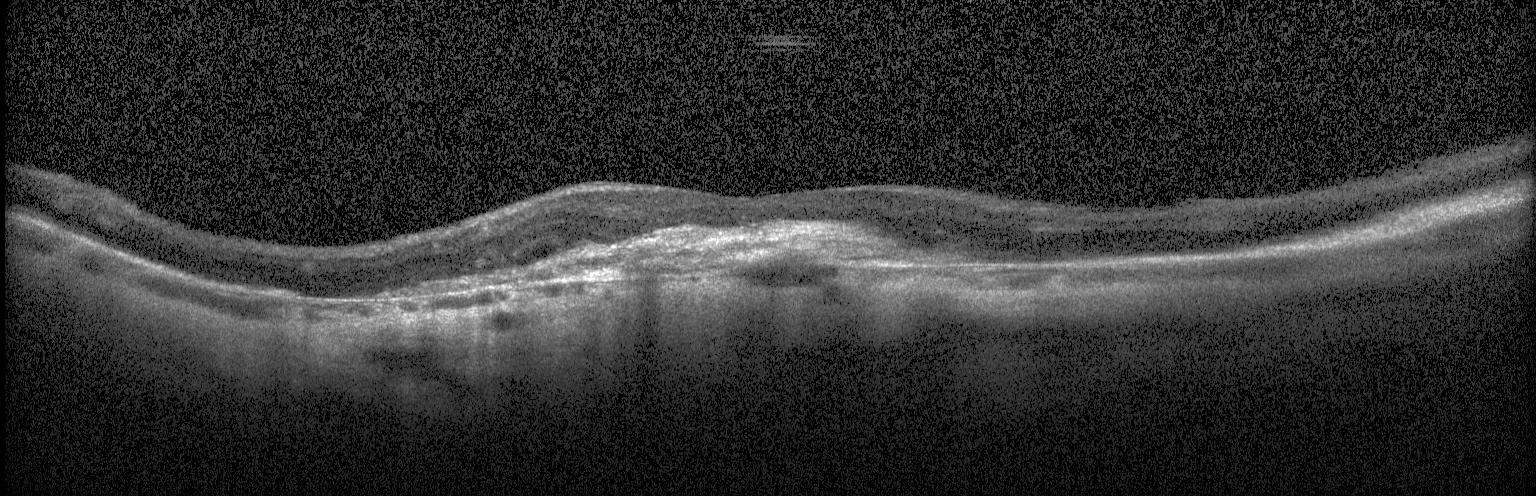 SD-OCT · OCT line scan. Finding: choroidal neovascularization (CNV).